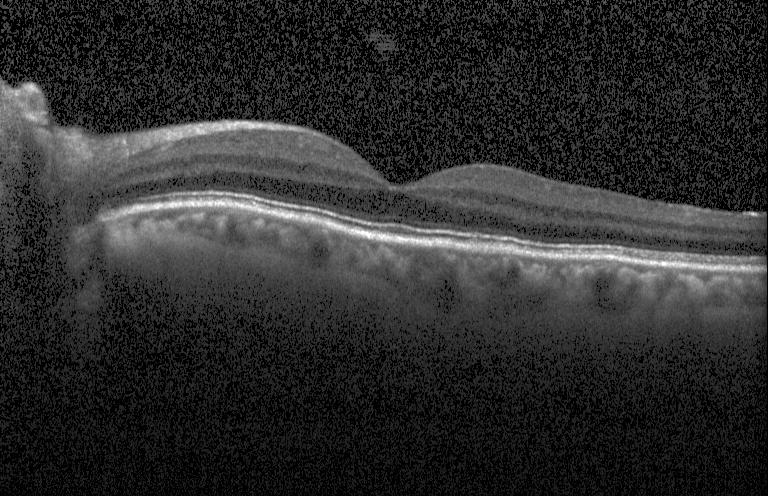

Dx: no choroidal neovascularization, diabetic macular edema, or drusen.